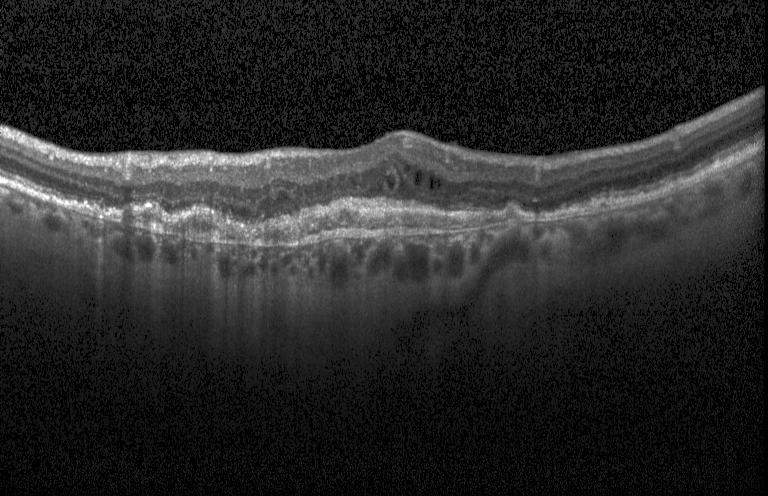

Finding: choroidal neovascularization.